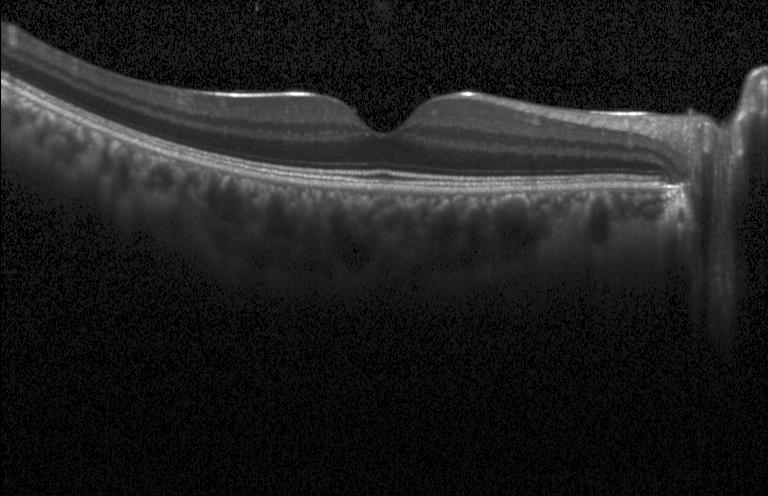

OCT scan showing no choroidal neovascularization, no diabetic macular edema, and no drusen.